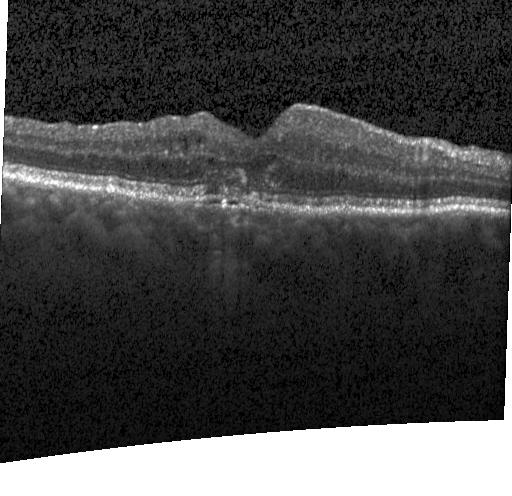 OCT finding: a choroidal neovascular membrane.